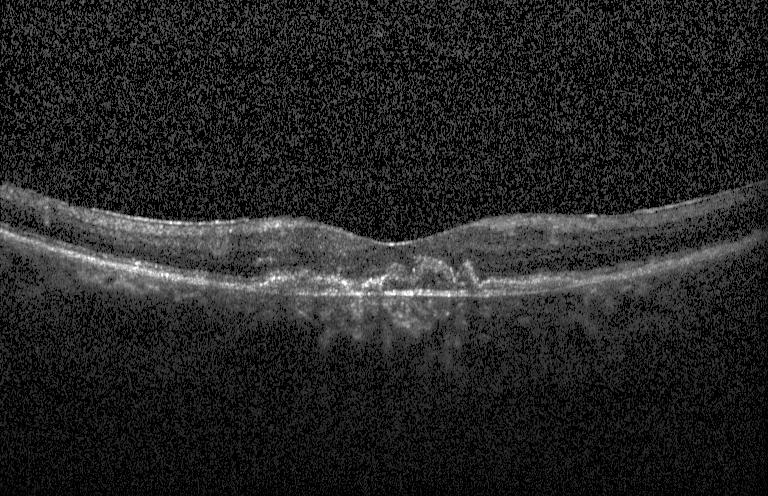

Acquired on a Heidelberg Spectralis · OCT B-scan · macular scan · SD-OCT.
OCT finding: CNV.